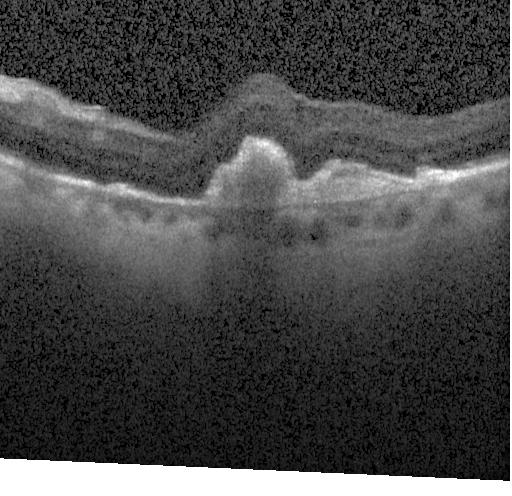 Spectral-domain optical coherence tomography. Optical coherence tomography scan
Diagnosis: choroidal neovascularization.